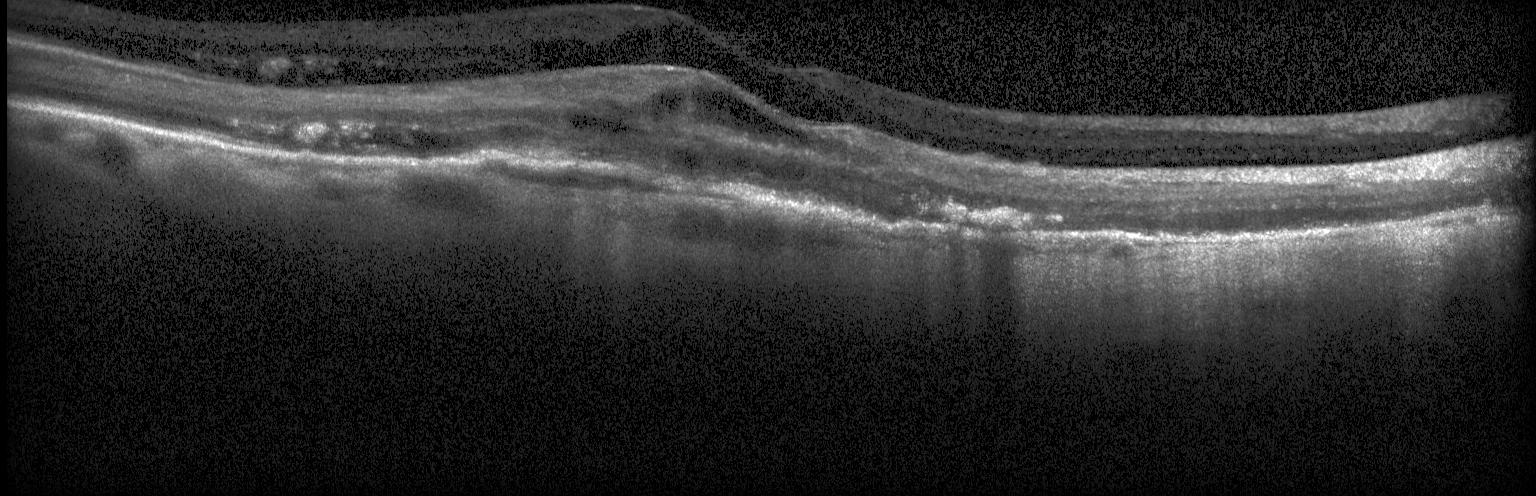 SD-OCT. Retinal OCT B-scan.
Dx: a choroidal neovascular membrane.